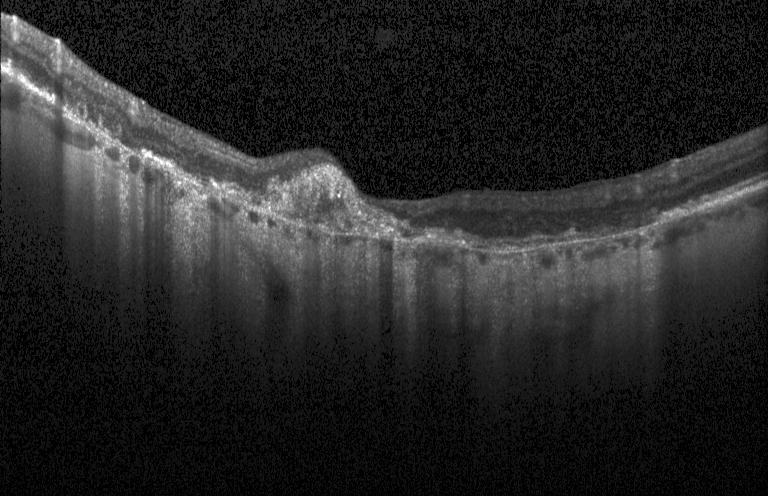 Centered on the fovea; optical coherence tomography scan.
The scan shows a choroidal neovascular membrane.